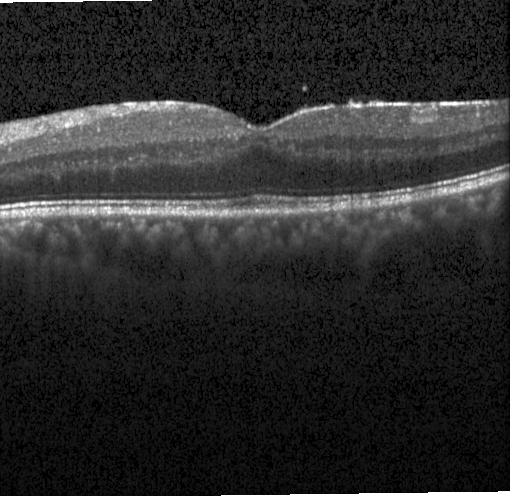

No CNV, DME, or drusen.